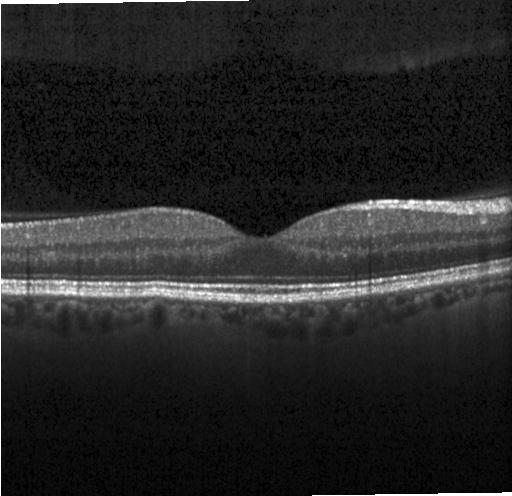
No evidence of choroidal neovascularization, diabetic macular edema, or drusen.